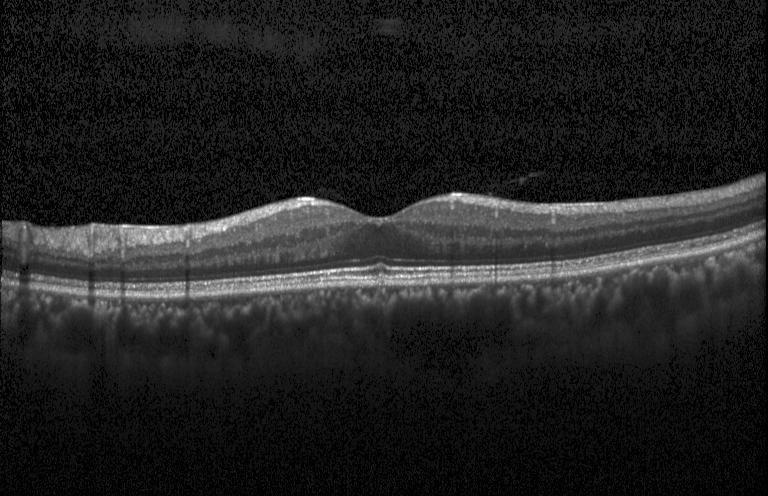 OCT line scan · spectral-domain optical coherence tomography
The scan shows no evidence of choroidal neovascularization, diabetic macular edema, or drusen.